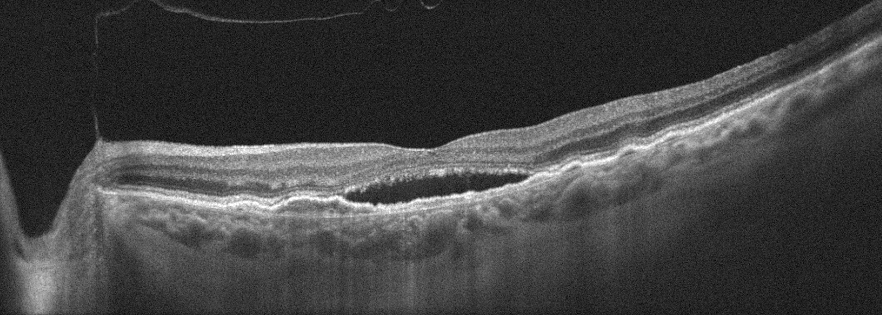
Retinal OCT B-scan · OS. OCT finding: AMD.